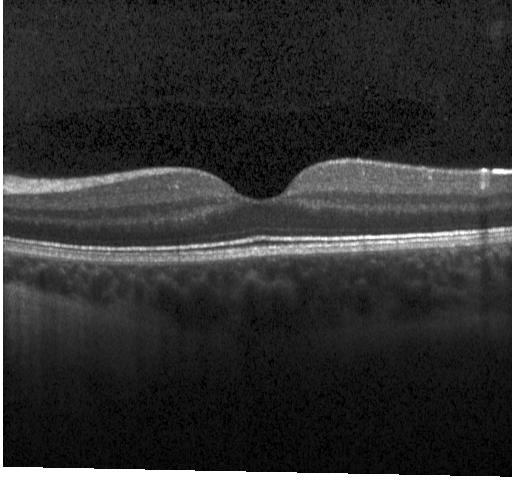
Acquired on a Heidelberg Spectralis, SD-OCT, OCT line scan, through the macula — Diagnosis: neither choroidal neovascularization, diabetic macular edema, nor drusen.